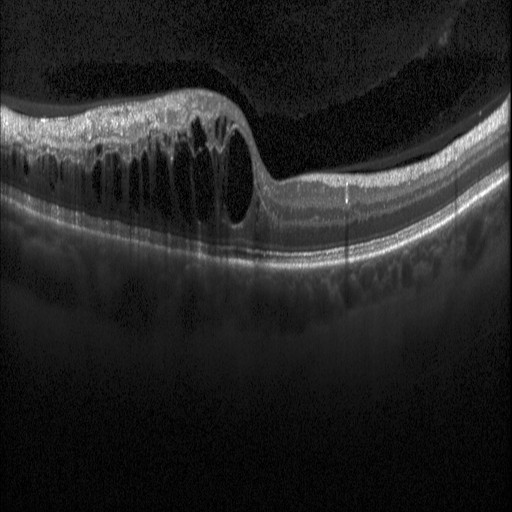 Optical coherence tomography scan — OCT finding: diabetic macular edema.